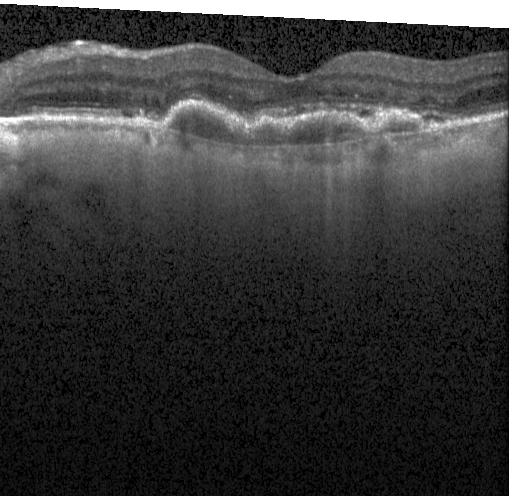
Heidelberg Spectralis OCT system. Optical coherence tomography scan
This B-scan demonstrates choroidal neovascularization.